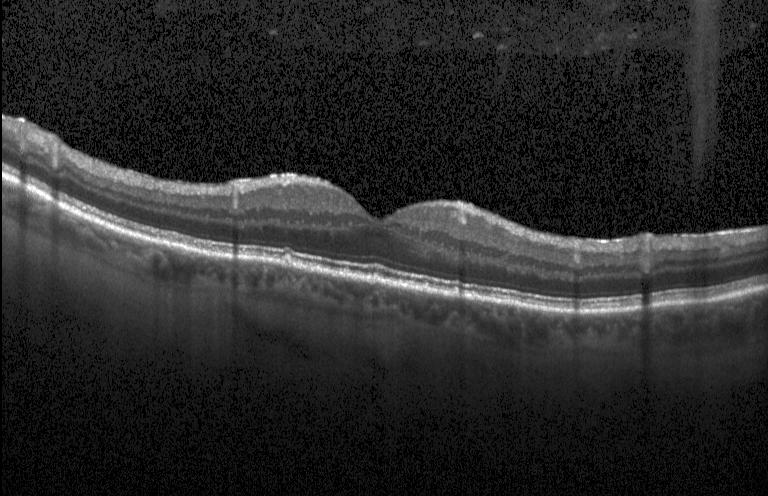 Finding: multiple drusen.